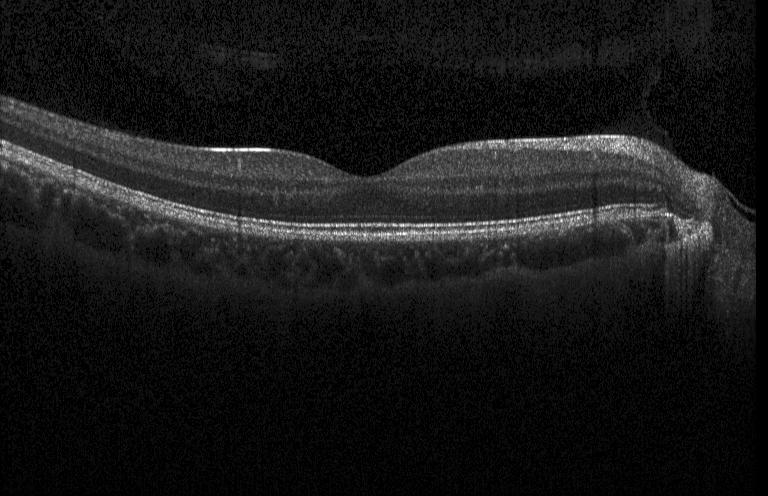 OCT line scan. Spectral-domain optical coherence tomography. Heidelberg Spectralis.
This B-scan demonstrates no evidence of choroidal neovascularization, diabetic macular edema, or drusen.